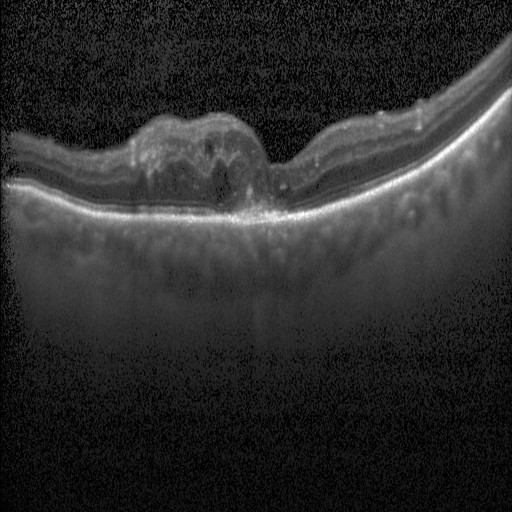

Macular OCT: DME.